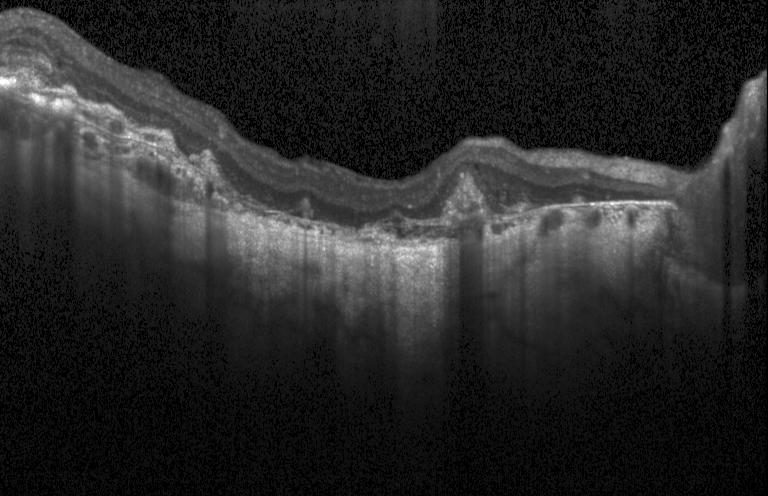 Retinal OCT cross-section showing a choroidal neovascular membrane.